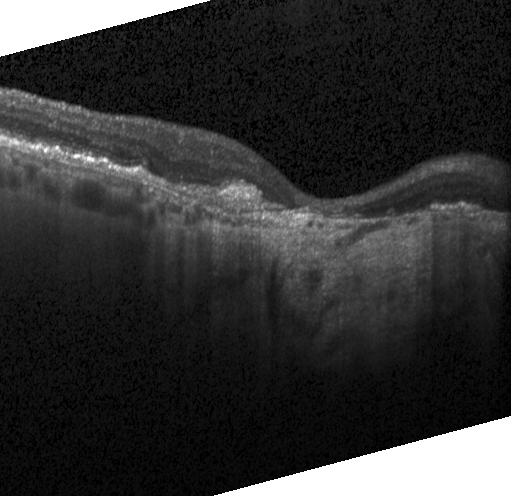
OCT line scan.
Assessment: a choroidal neovascular membrane.